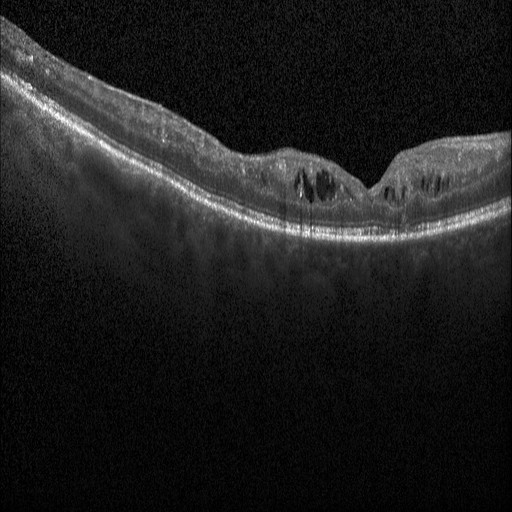

OCT finding: diabetic macular edema.